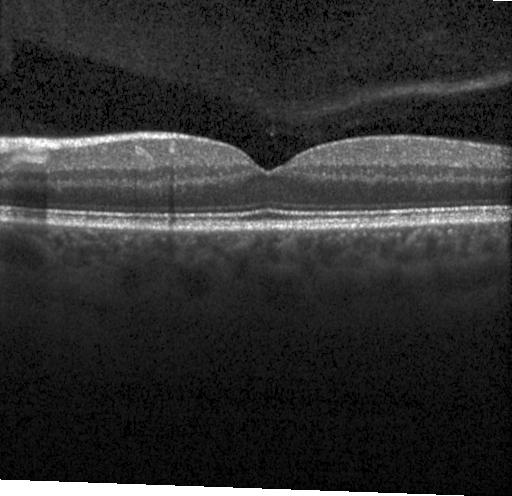 Spectral-domain OCT, OCT line scan, through the macula. Diagnosis: no CNV, DME, or drusen.